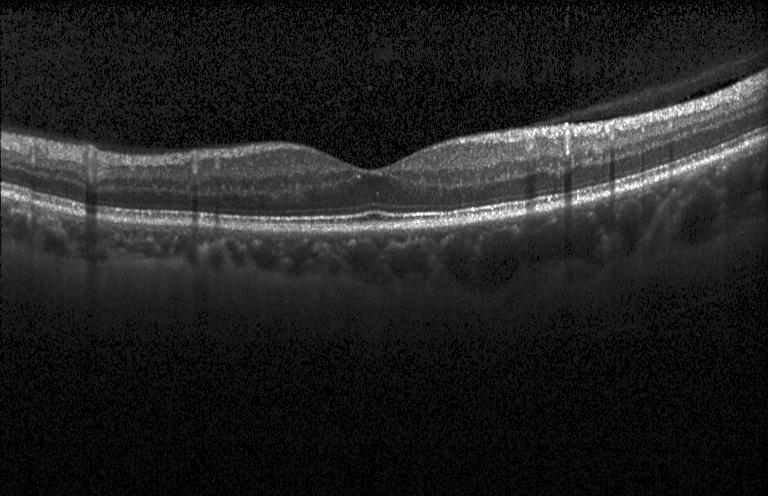

Fovea-centered · OCT B-scan
Finding: neither choroidal neovascularization, diabetic macular edema, nor drusen.